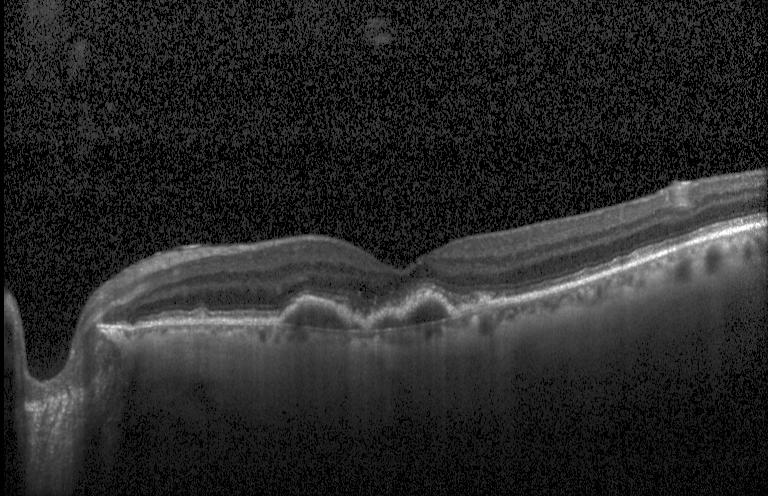
Retinal OCT cross-section · acquired on a Heidelberg Spectralis · SD-OCT
OCT finding: CNV.